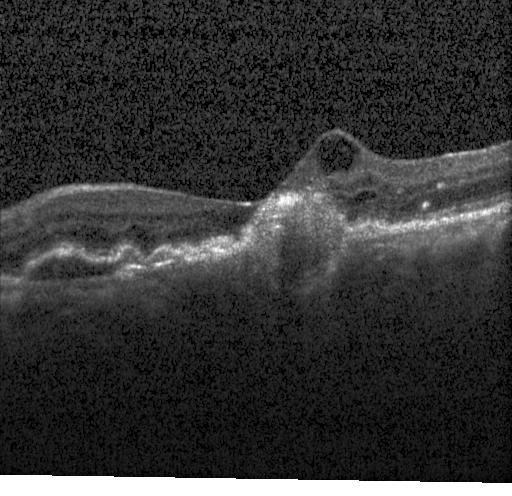
OCT B-scan. Spectral-domain OCT. Instrument: Heidelberg Spectralis — Assessment: a choroidal neovascular membrane.